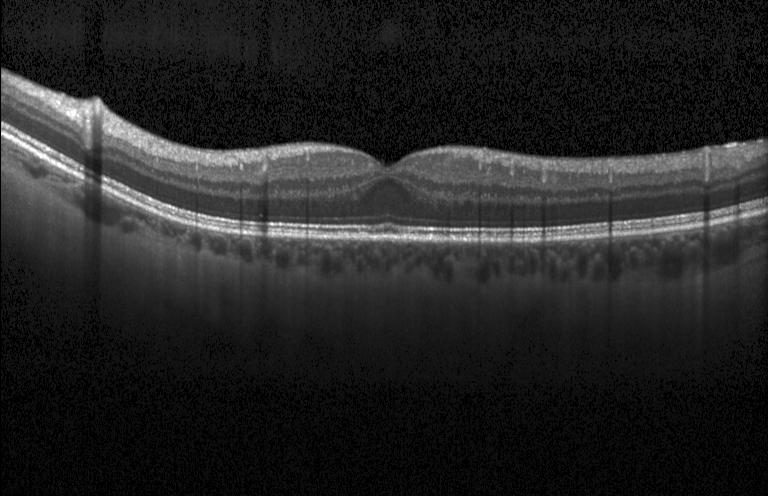
Retinal OCT cross-section. Spectral-domain OCT. Centered on the fovea. Instrument: Heidelberg Spectralis — The scan shows no choroidal neovascularization, diabetic macular edema, or drusen.